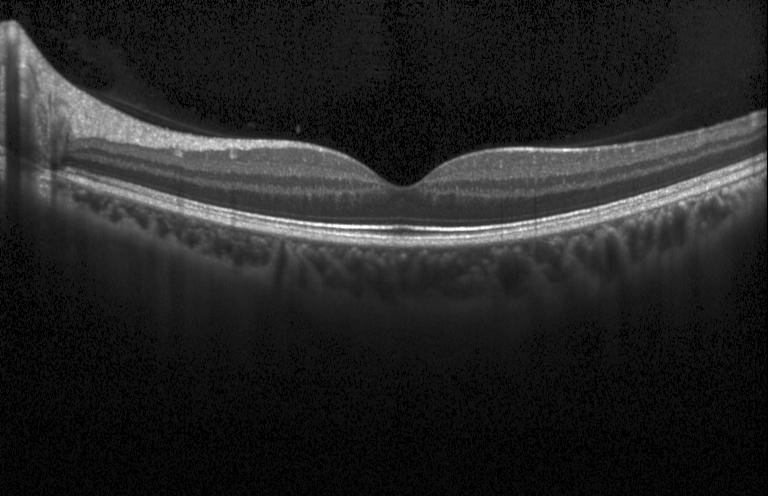

Through the macula; spectral-domain OCT; retinal OCT B-scan; acquired on a Heidelberg Spectralis
Assessment: no CNV, no DME, and no drusen.